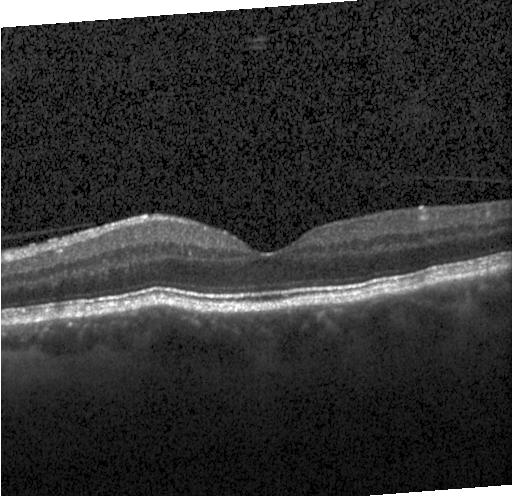
Spectral-domain optical coherence tomography, fovea-centered, retinal OCT cross-section, instrument: Heidelberg Spectralis. Dx: no choroidal neovascularization, diabetic macular edema, or drusen.